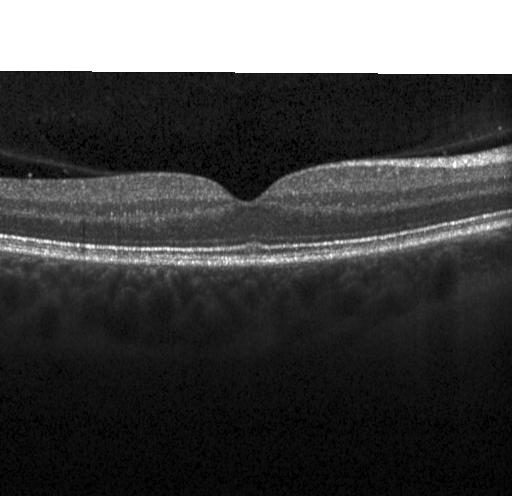

SD-OCT, OCT line scan, acquired on a Heidelberg Spectralis.
Impression: neither choroidal neovascularization, diabetic macular edema, nor drusen.